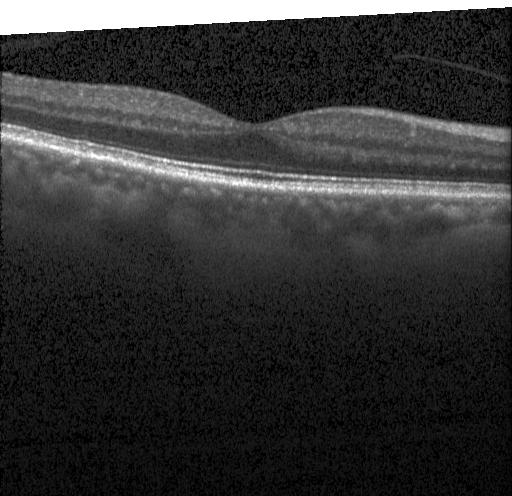 OCT finding: no evidence of choroidal neovascularization, diabetic macular edema, or drusen.